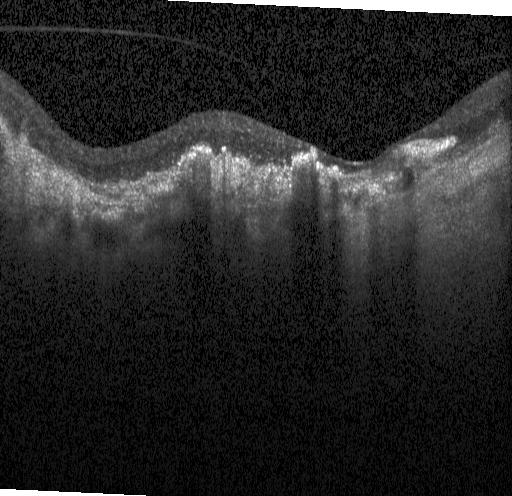

OCT finding: choroidal neovascularization.